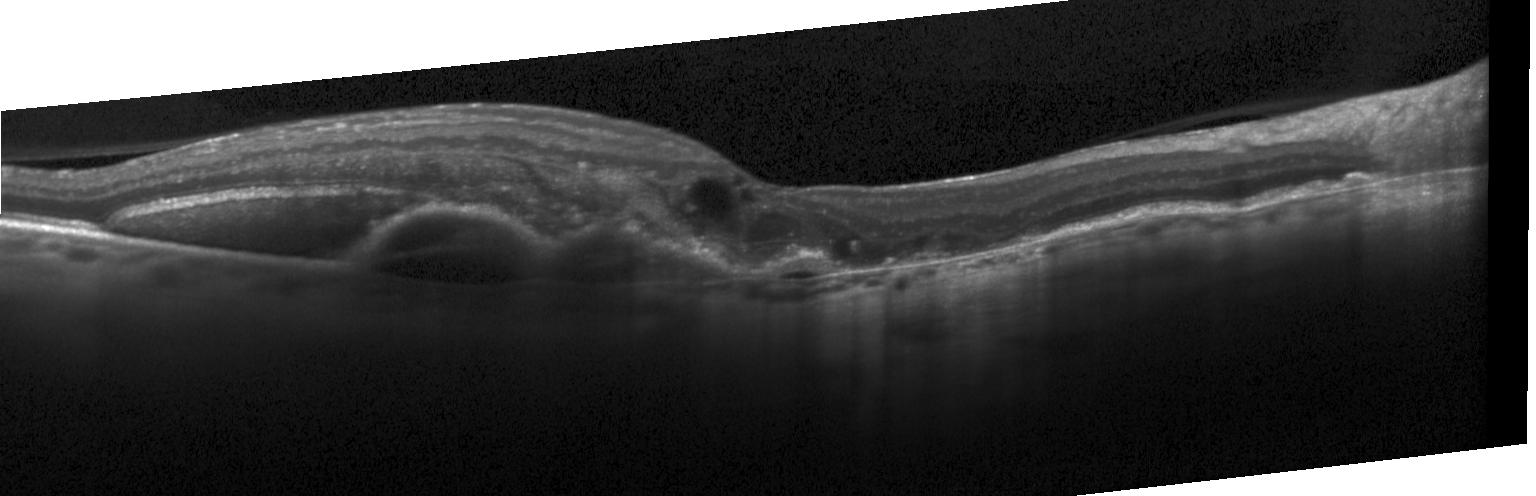

OCT scan showing choroidal neovascularization (CNV).